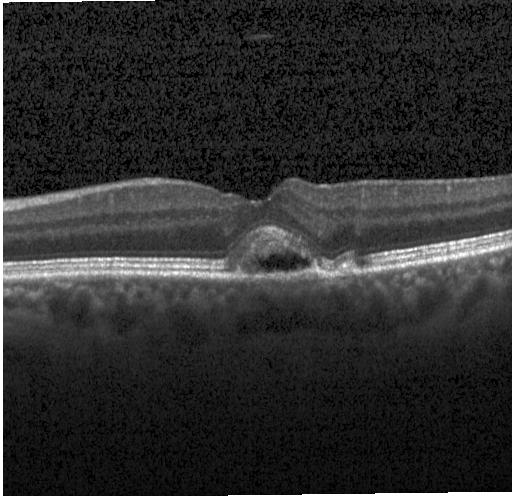
Heidelberg Spectralis; OCT B-scan; SD-OCT.
This B-scan demonstrates CNV.